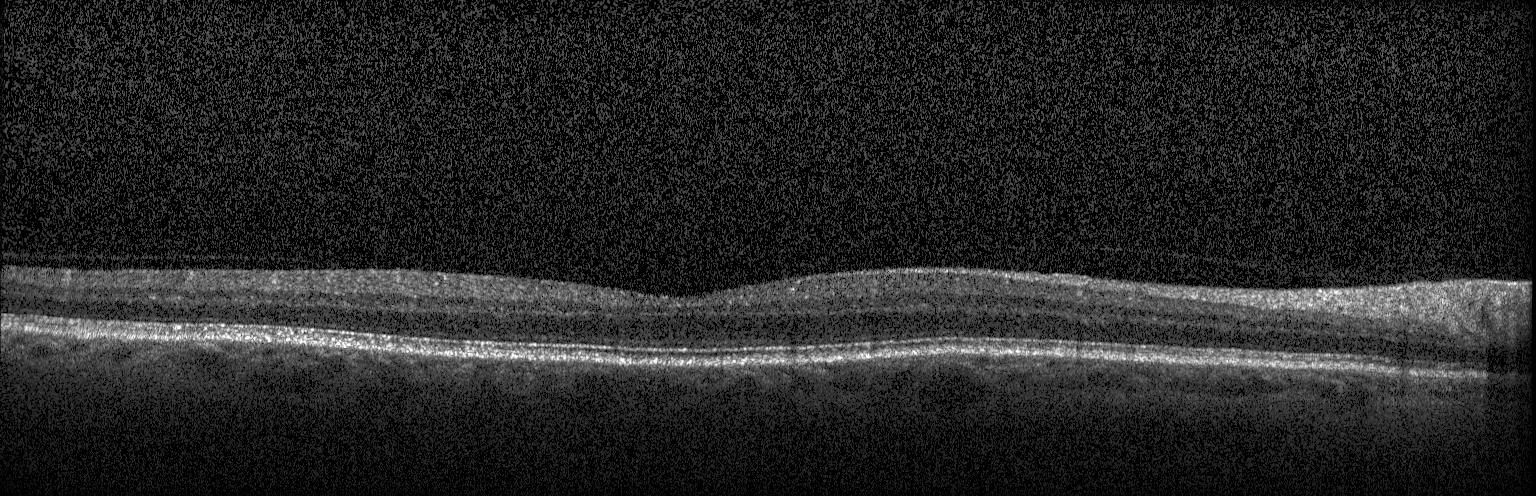 Instrument: Heidelberg Spectralis, fovea-centered, spectral-domain OCT, optical coherence tomography scan — Impression: neither CNV, DME, nor drusen.